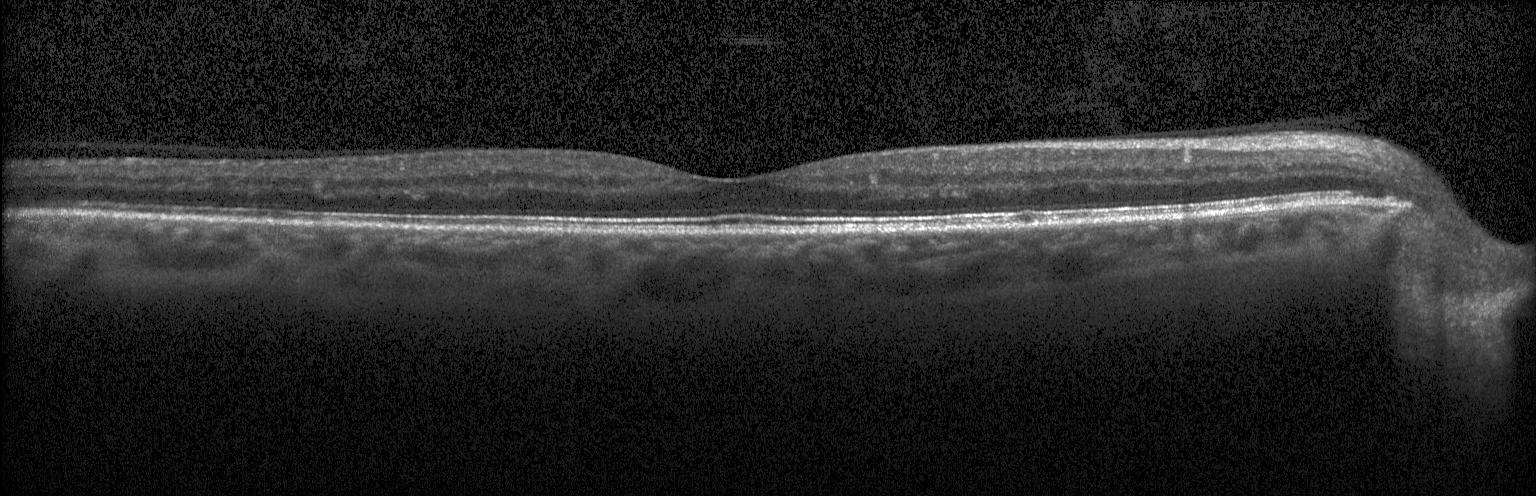 Heidelberg Spectralis; OCT B-scan
Macular OCT: neither choroidal neovascularization, diabetic macular edema, nor drusen.